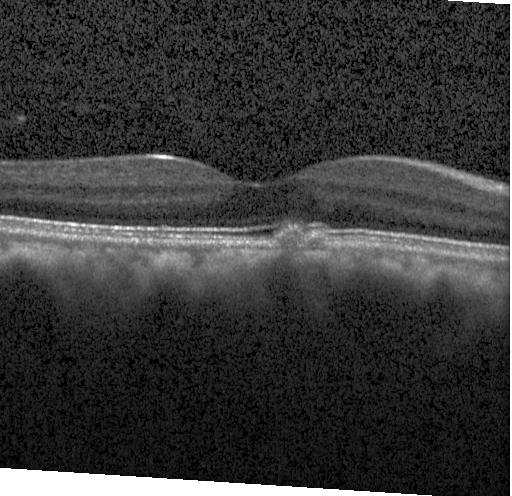

Retinal OCT cross-section.
Finding: sub-RPE drusenoid deposits.